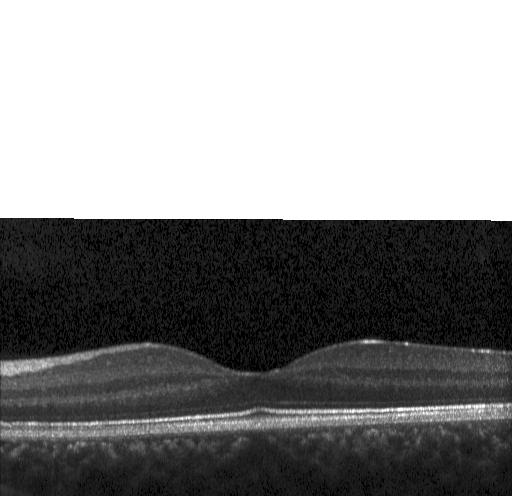

Heidelberg Spectralis; spectral-domain optical coherence tomography; retinal OCT B-scan; centered on the fovea — Dx: no evidence of choroidal neovascularization, diabetic macular edema, or drusen.